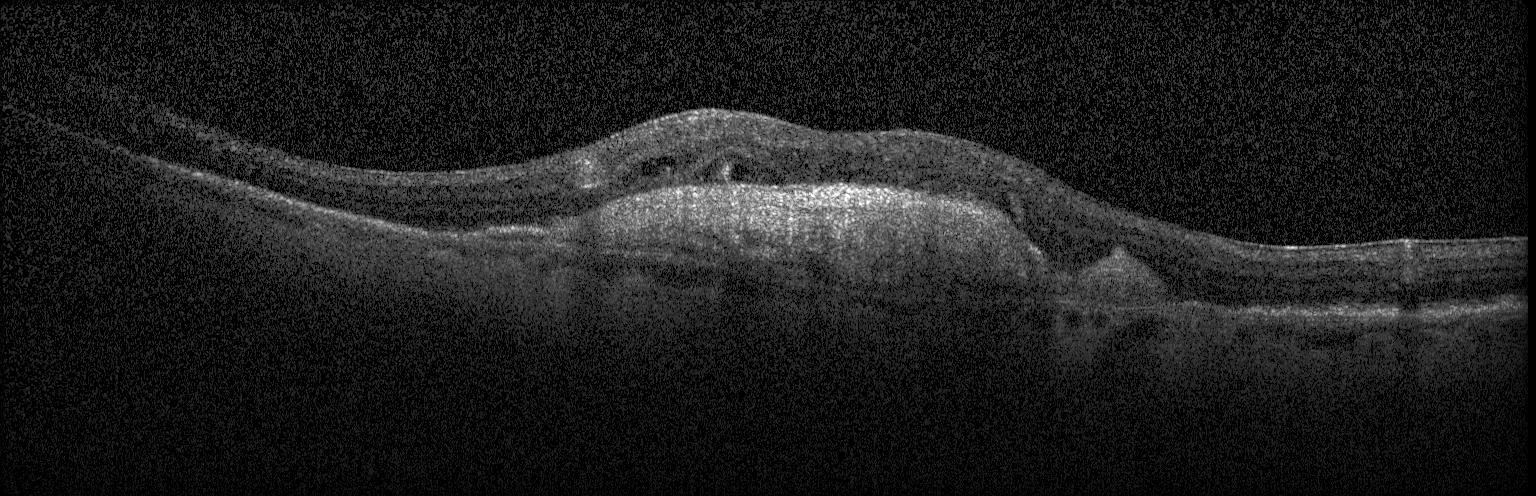

OCT scan showing a choroidal neovascular membrane.